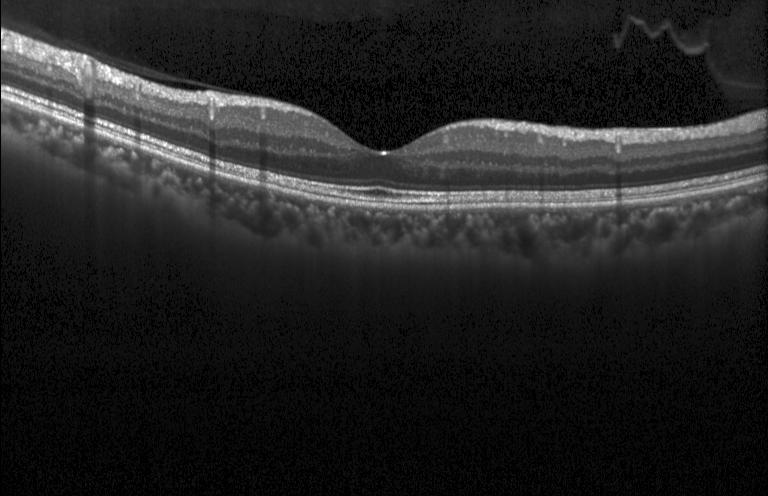 OCT finding: no choroidal neovascularization, diabetic macular edema, or drusen.